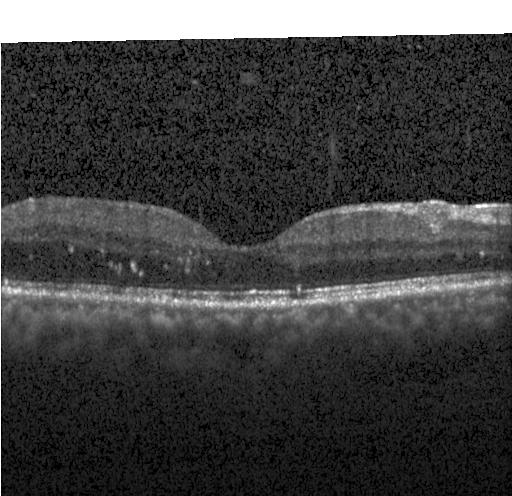

OCT line scan · acquired on a Heidelberg Spectralis · through the macula · spectral-domain optical coherence tomography — Diagnosis: diabetic macular edema (DME).